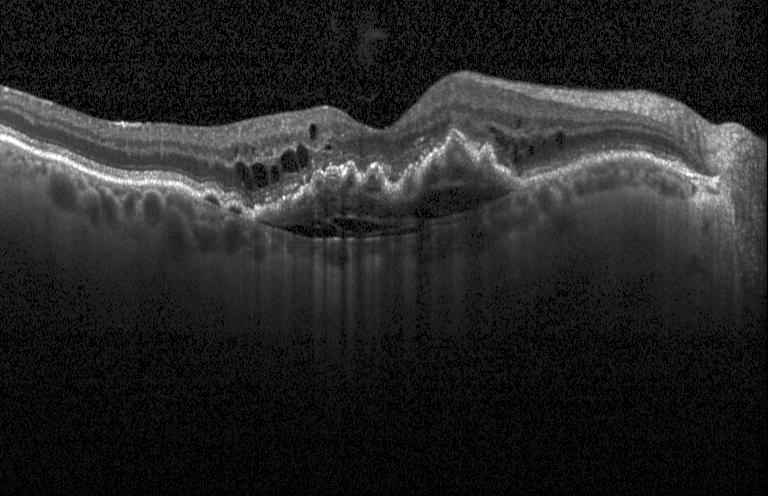

Heidelberg Spectralis OCT system; through the macula; OCT B-scan
Choroidal neovascularization.